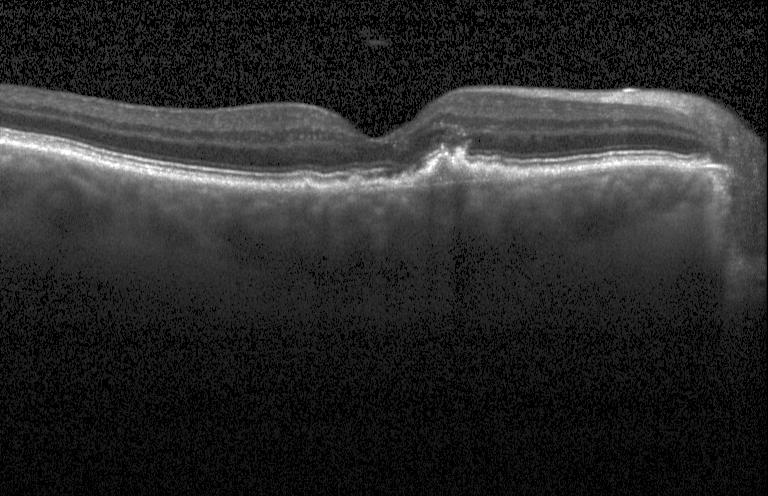

This B-scan demonstrates a choroidal neovascular membrane.